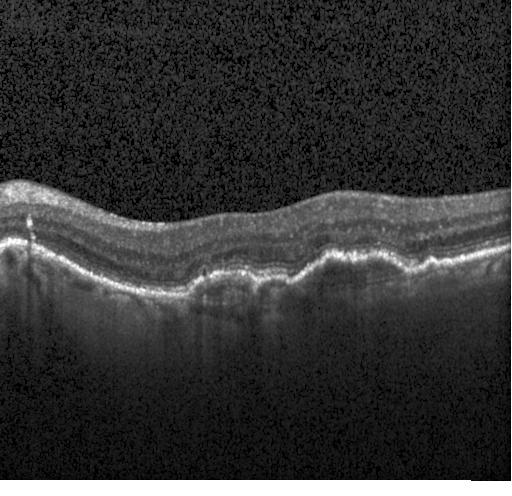 Optical coherence tomography scan. Diagnosis: choroidal neovascularization.